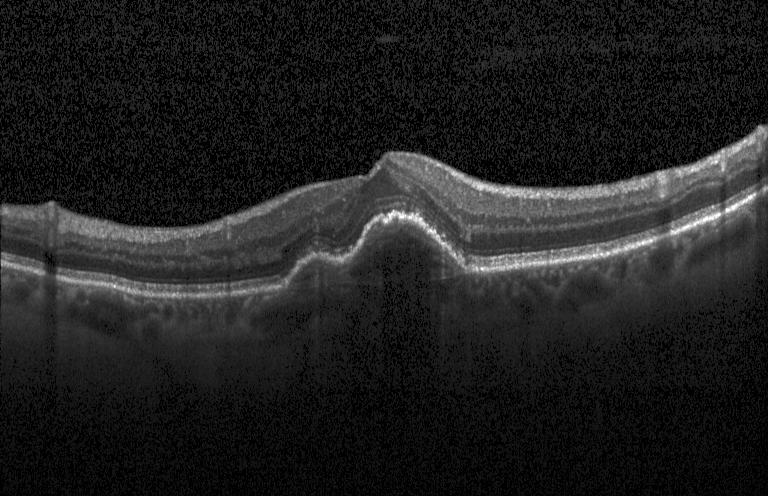

Horizontal scan through the fovea, retinal OCT cross-section — Impression: a choroidal neovascular membrane.